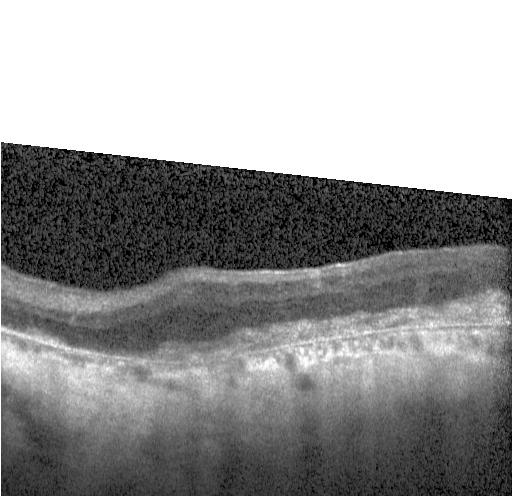 Heidelberg Spectralis, SD-OCT, retinal OCT cross-section — This B-scan demonstrates choroidal neovascularization.